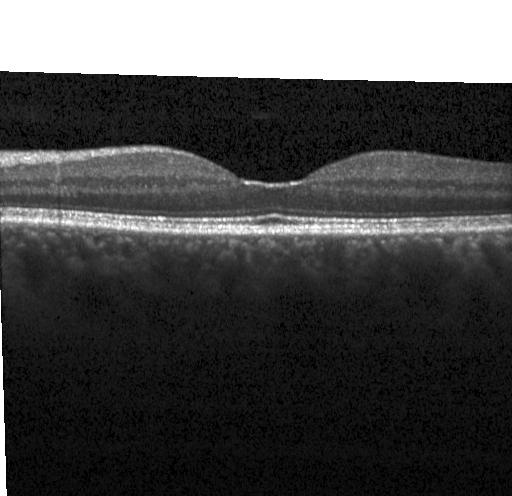

Finding: no choroidal neovascularization, no diabetic macular edema, and no drusen.